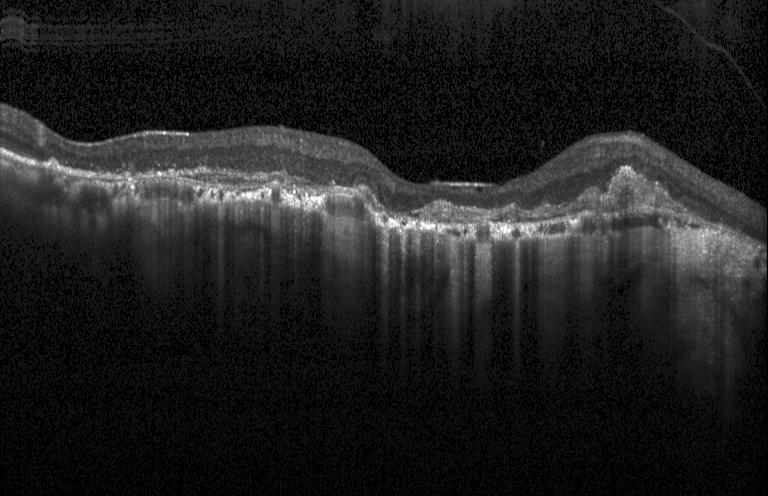

Finding: a choroidal neovascular membrane.